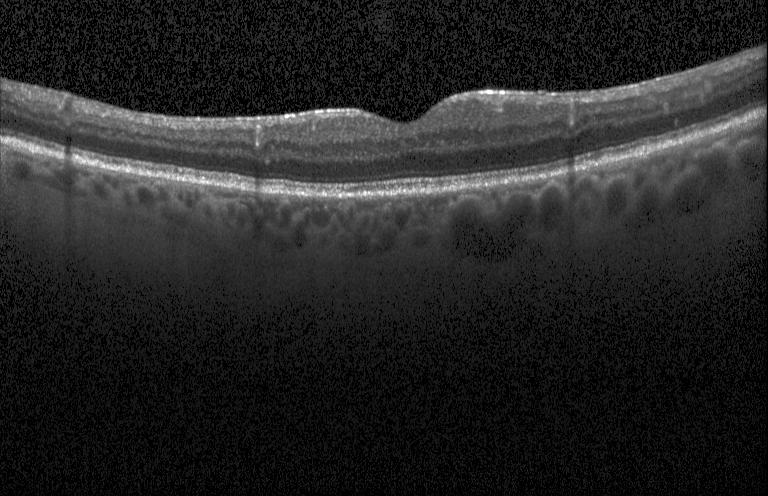 Impression: no evidence of choroidal neovascularization, diabetic macular edema, or drusen.